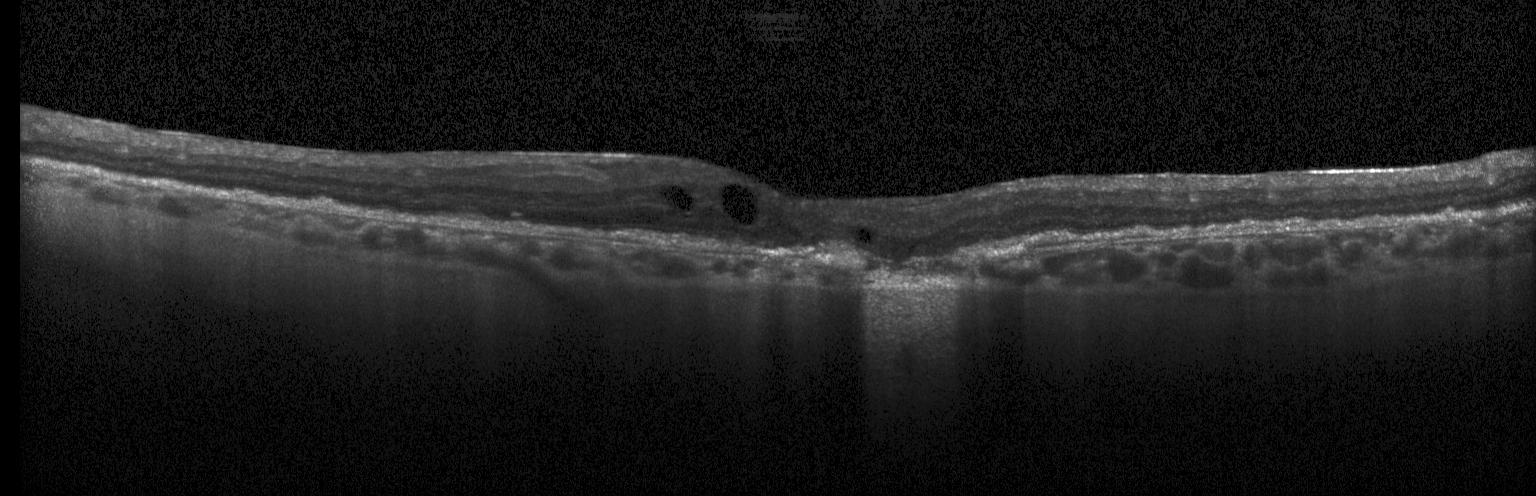
OCT scan showing CNV.